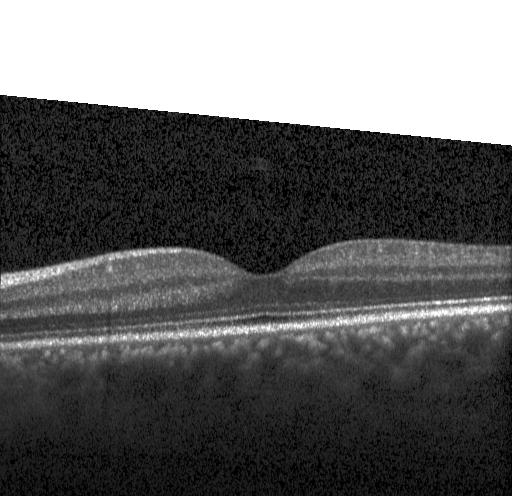

OCT finding: no choroidal neovascularization, no diabetic macular edema, and no drusen.